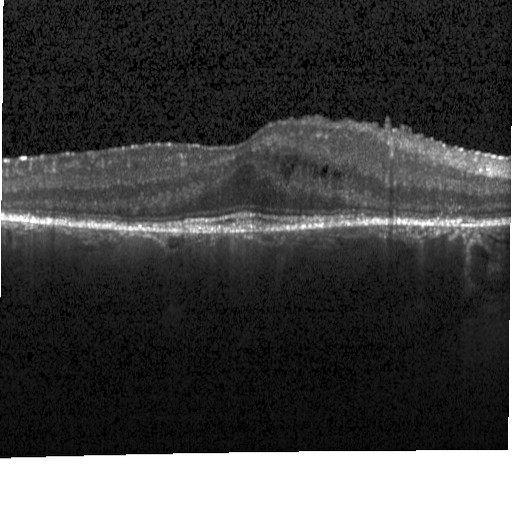 Optical coherence tomography B-scan — Finding: diabetic macular edema.